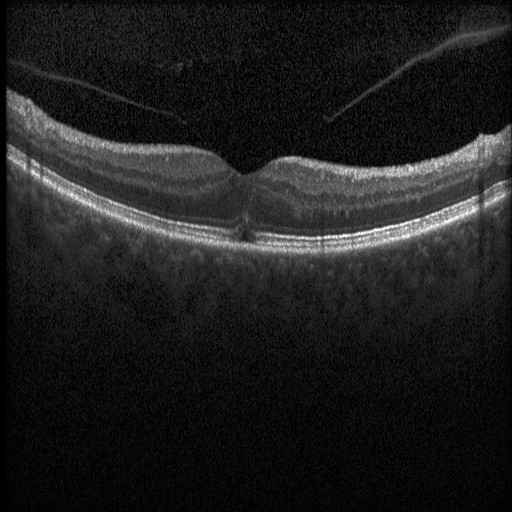 OCT line scan. Diagnosis: diabetic macular edema.